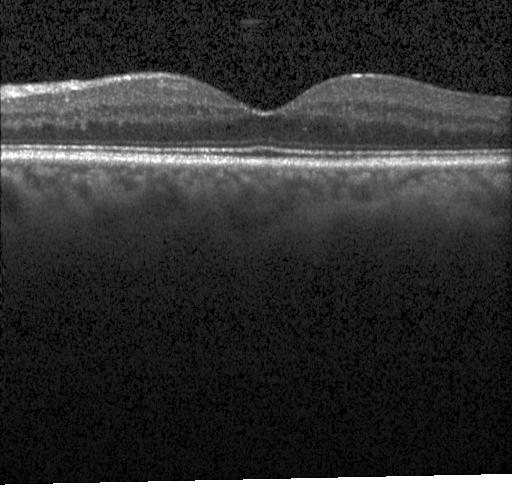
Diagnosis: no evidence of CNV, DME, or drusen.